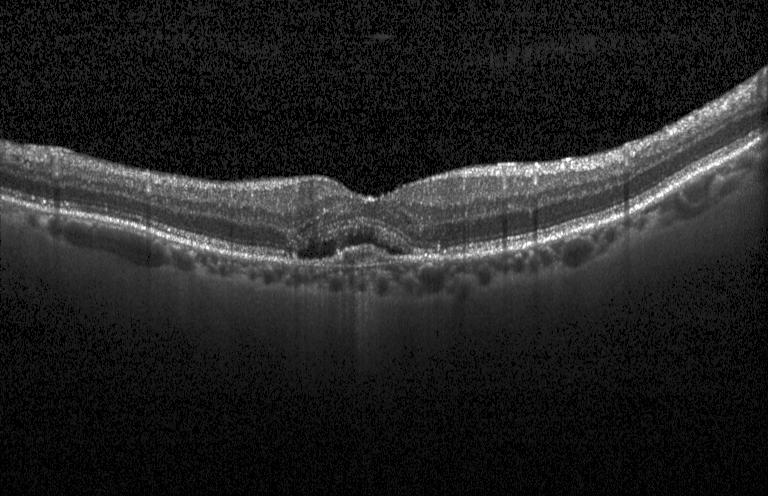
Retinal OCT cross-section · spectral-domain OCT
Diagnosis: a choroidal neovascular membrane.